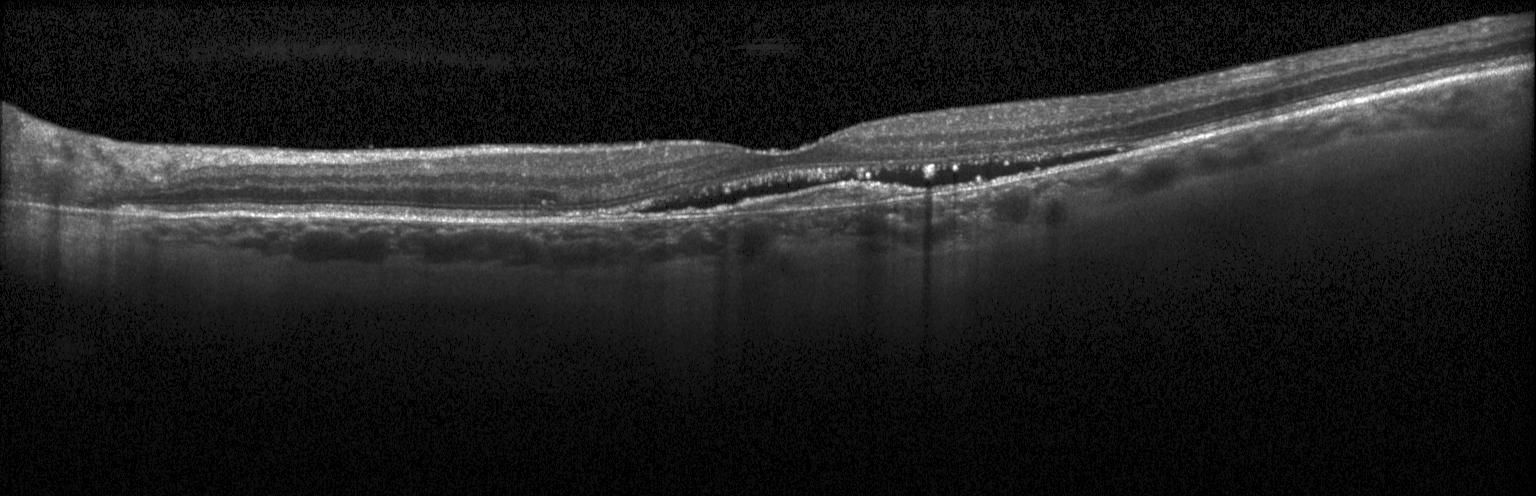 Impression: CNV.